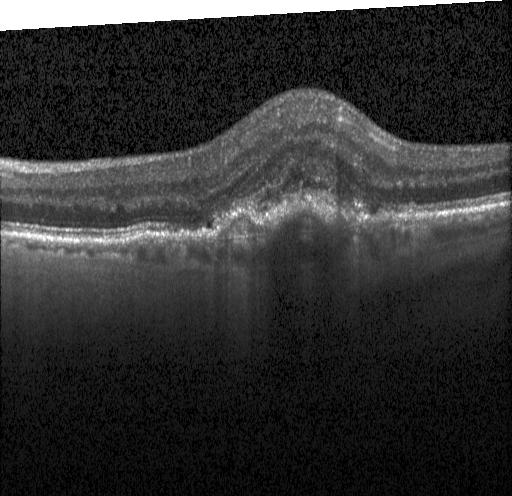
Finding: a choroidal neovascular membrane.